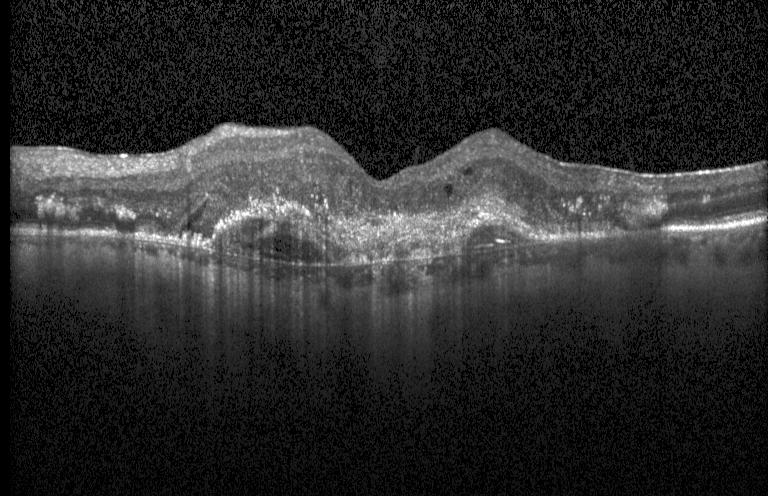
Acquired on a Heidelberg Spectralis · optical coherence tomography B-scan.
Dx: a choroidal neovascular membrane.